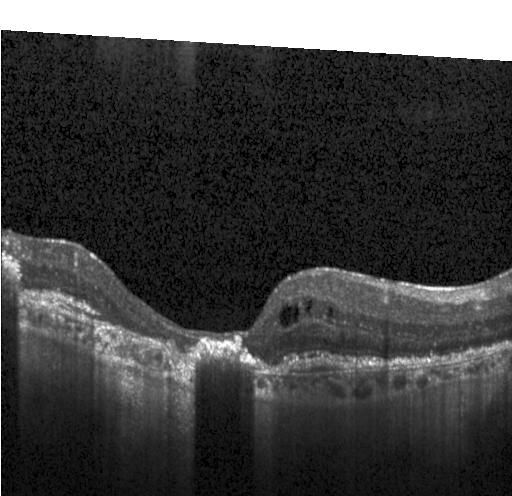 Finding: a choroidal neovascular membrane.